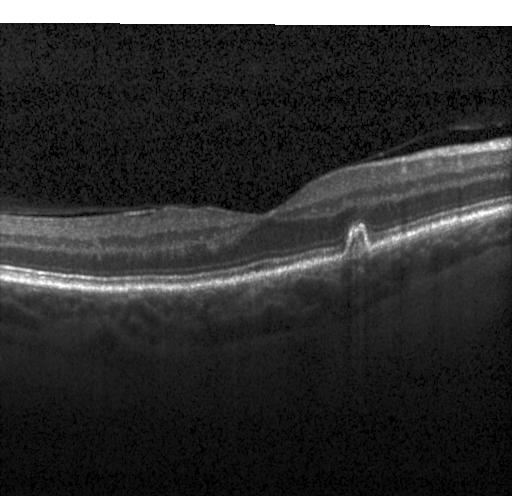
Dx: drusen.